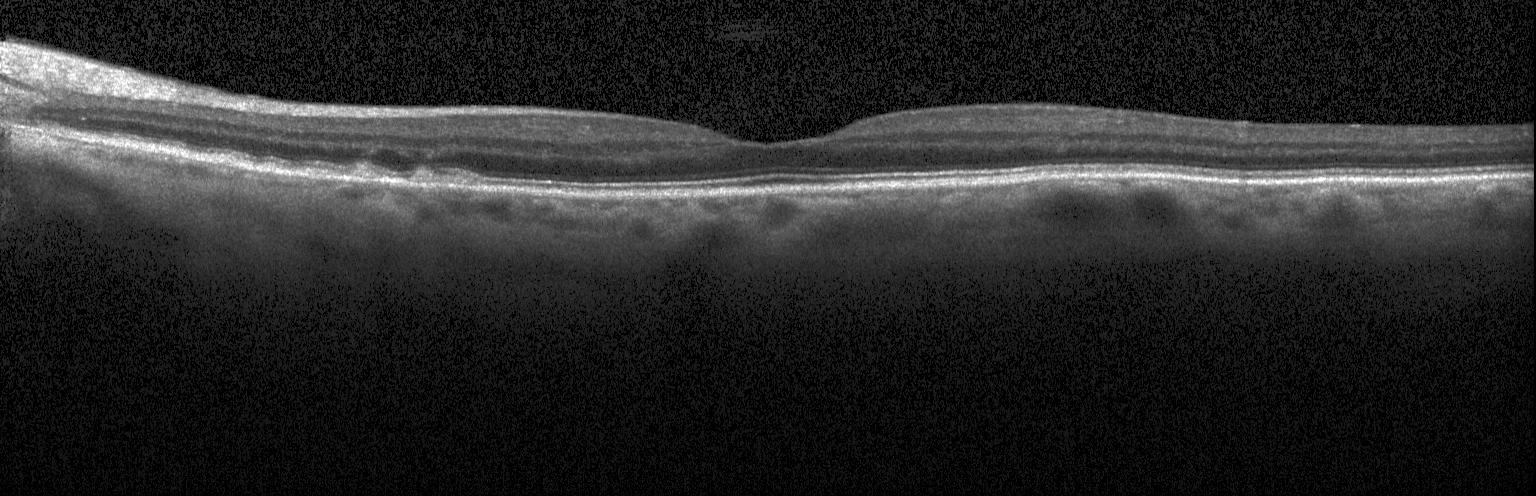

Retinal OCT B-scan. SD-OCT. Heidelberg Spectralis
Dx: multiple drusen.